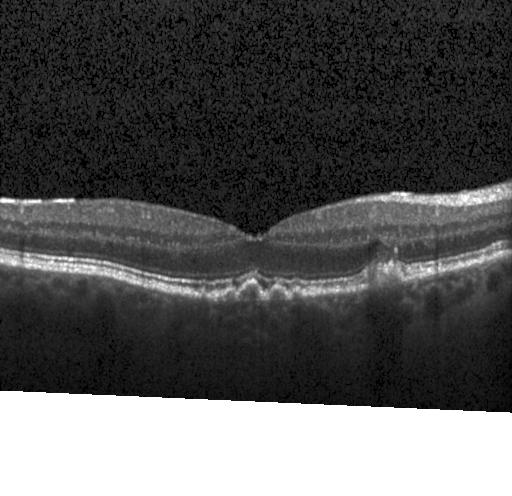
Heidelberg Spectralis OCT system. Optical coherence tomography scan. This B-scan demonstrates CNV.